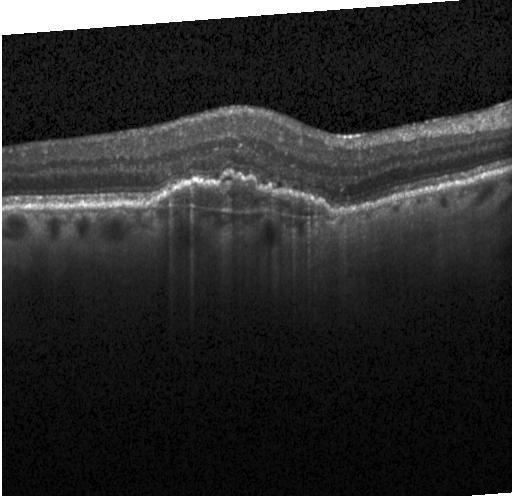 OCT scan showing choroidal neovascularization.